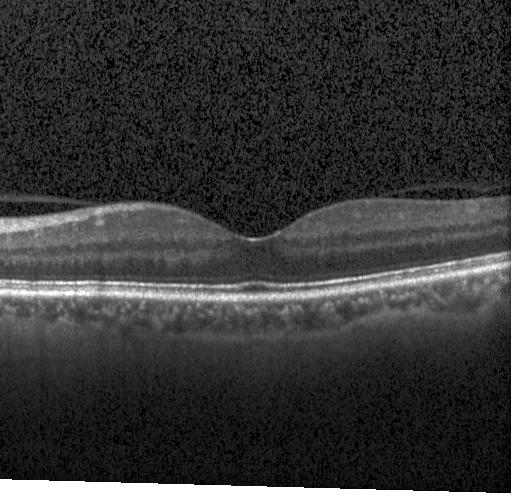
SD-OCT. Optical coherence tomography scan — No evidence of choroidal neovascularization, diabetic macular edema, or drusen.